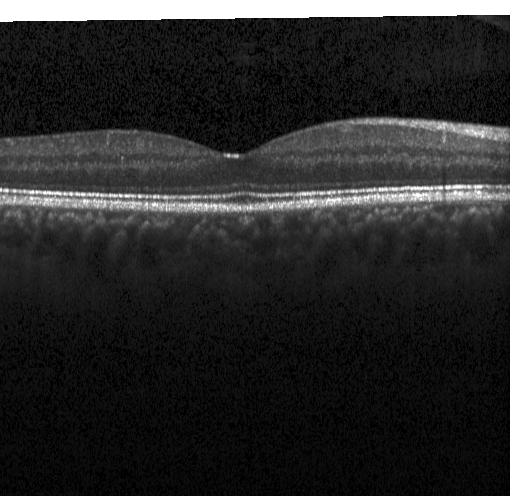
Macular OCT: no evidence of choroidal neovascularization, diabetic macular edema, or drusen.